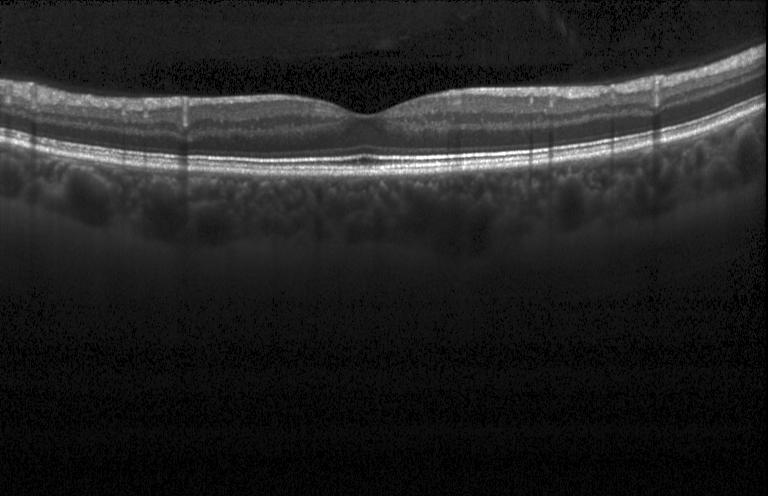
Neither choroidal neovascularization, diabetic macular edema, nor drusen.